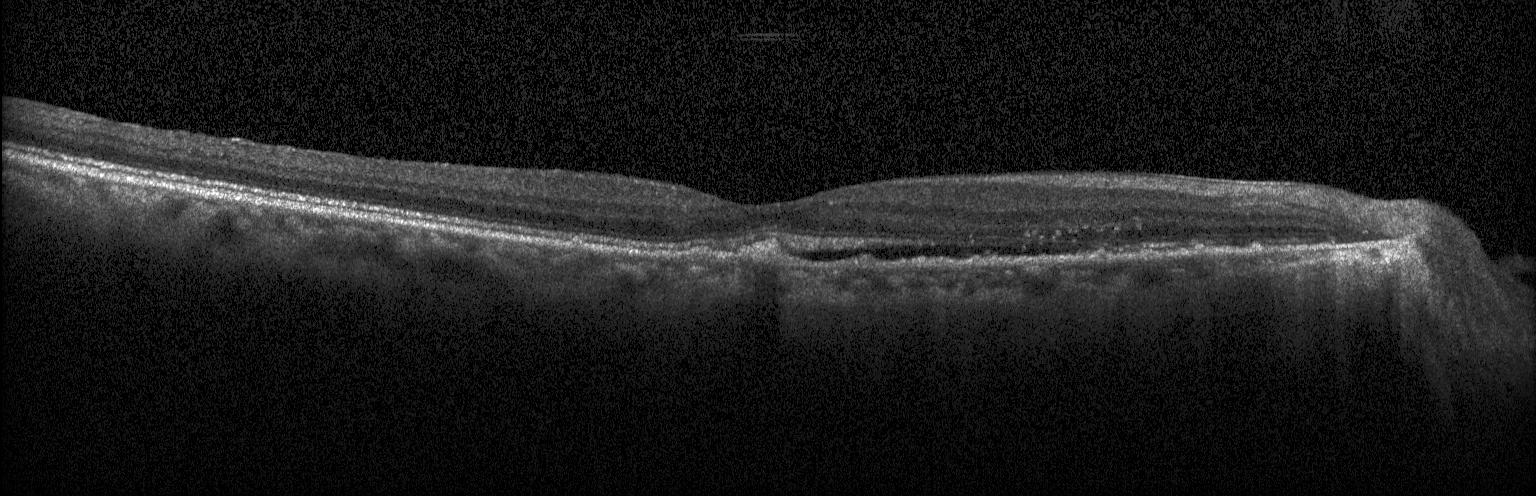 Optical coherence tomography B-scan.
Assessment: a choroidal neovascular membrane.